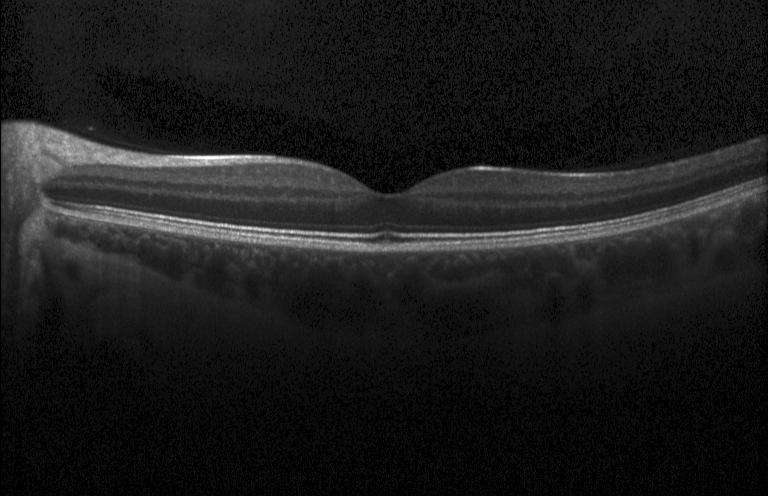 OCT B-scan
Diagnosis: no choroidal neovascularization, no diabetic macular edema, and no drusen.